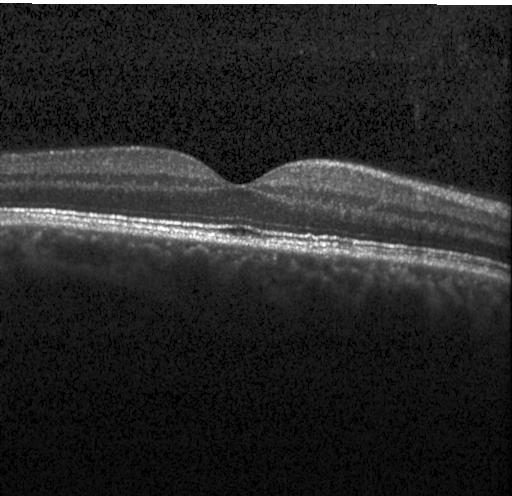

Acquired on a Heidelberg Spectralis. OCT B-scan. SD-OCT — Impression: no choroidal neovascularization, no diabetic macular edema, and no drusen.